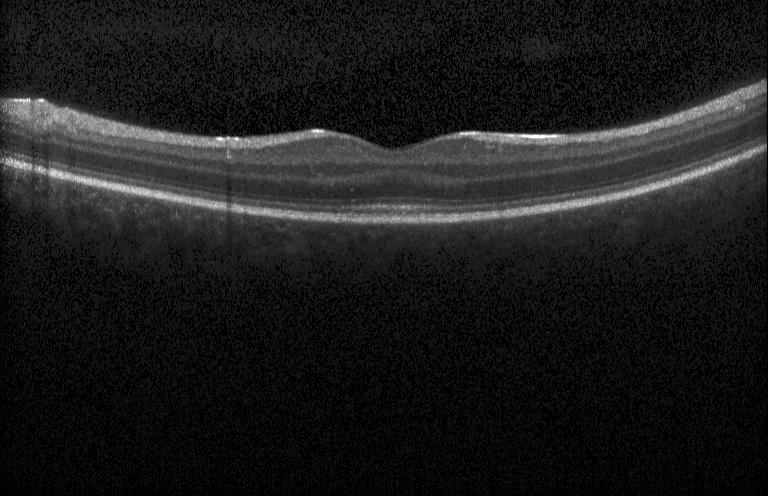
OCT line scan.
Finding: no choroidal neovascularization, no diabetic macular edema, and no drusen.